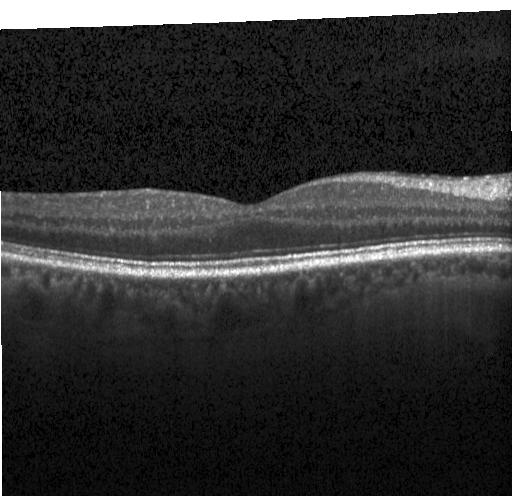
OCT B-scan showing no CNV, DME, or drusen.